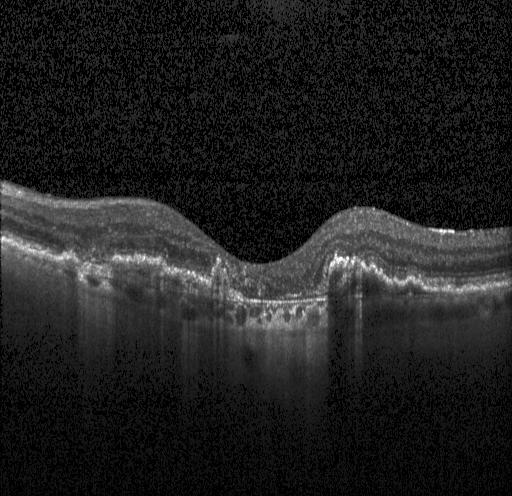 Retinal OCT B-scan. Heidelberg Spectralis. SD-OCT — Diagnosis: choroidal neovascularization.